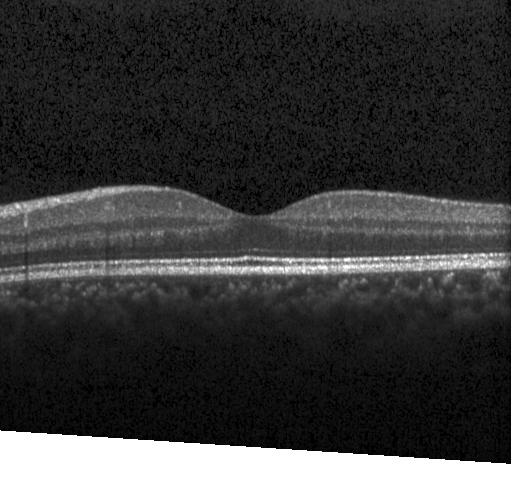
Heidelberg Spectralis. Optical coherence tomography B-scan
Neither CNV, DME, nor drusen.